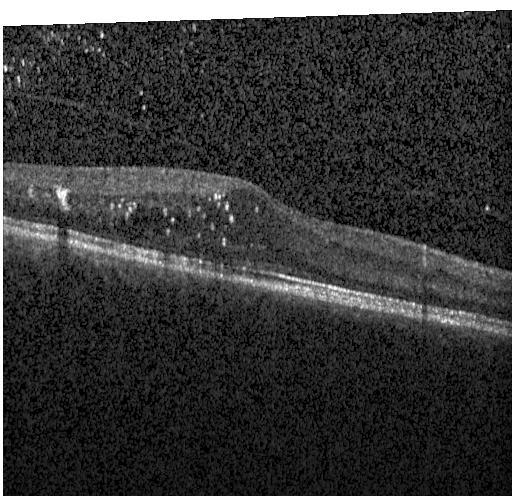
Spectral-domain optical coherence tomography, retinal OCT B-scan, through the macula — Impression: diabetic macular edema.